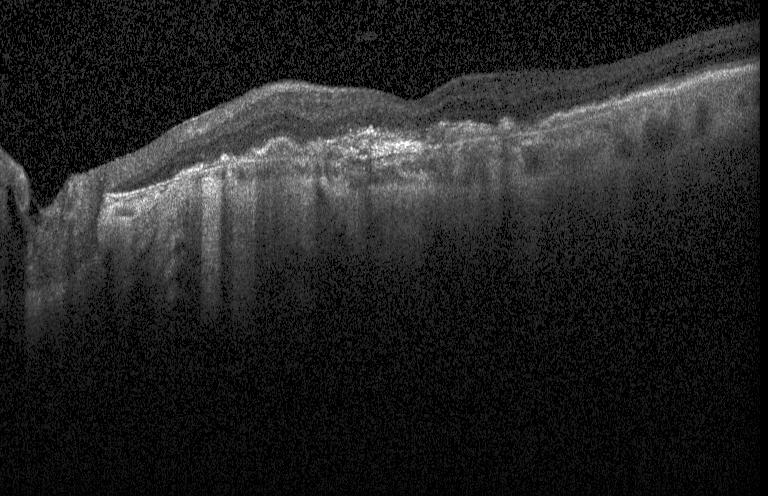
Diagnosis: CNV.